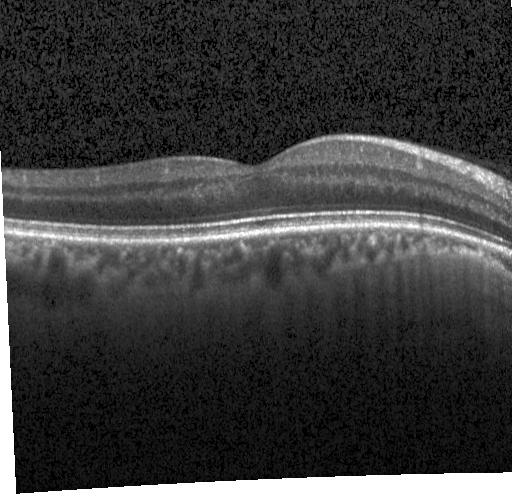
Diagnosis: no CNV, DME, or drusen.